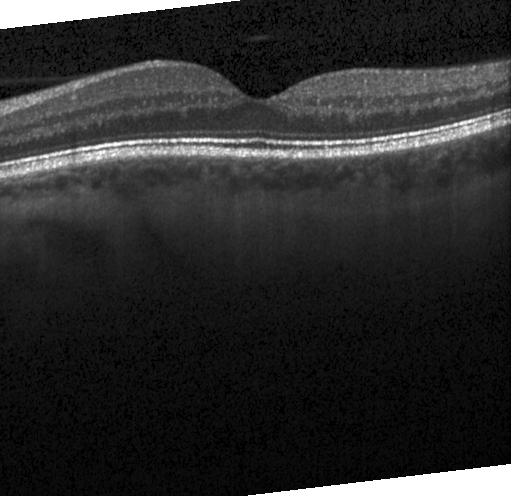 OCT B-scan
Diagnosis: no choroidal neovascularization, no diabetic macular edema, and no drusen.